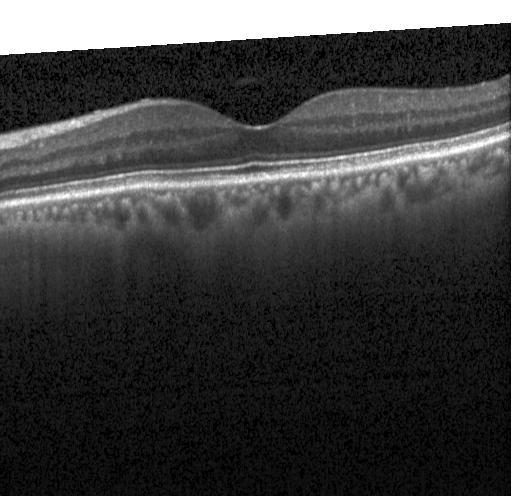 Dx: no choroidal neovascularization, diabetic macular edema, or drusen.